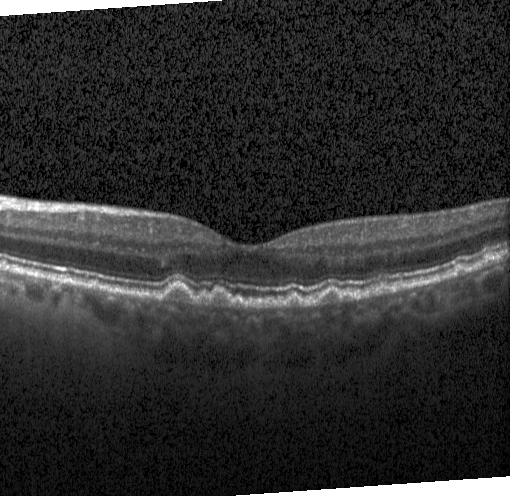 OCT B-scan — Diagnosis: drusen.